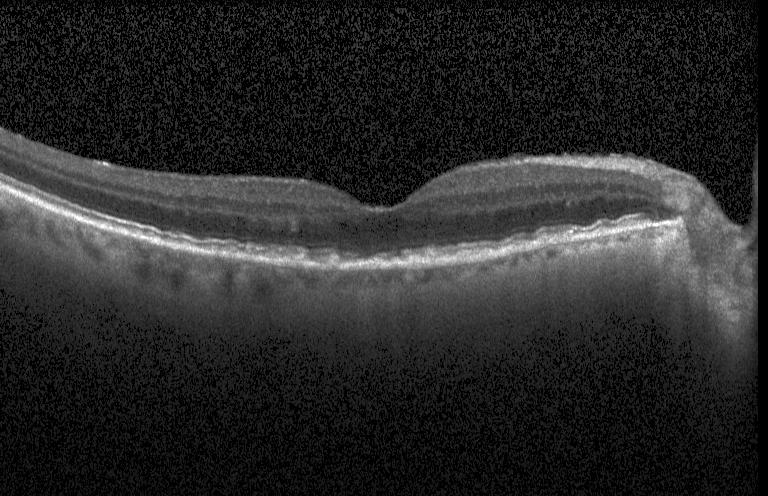

Retinal OCT B-scan
Finding: drusen.